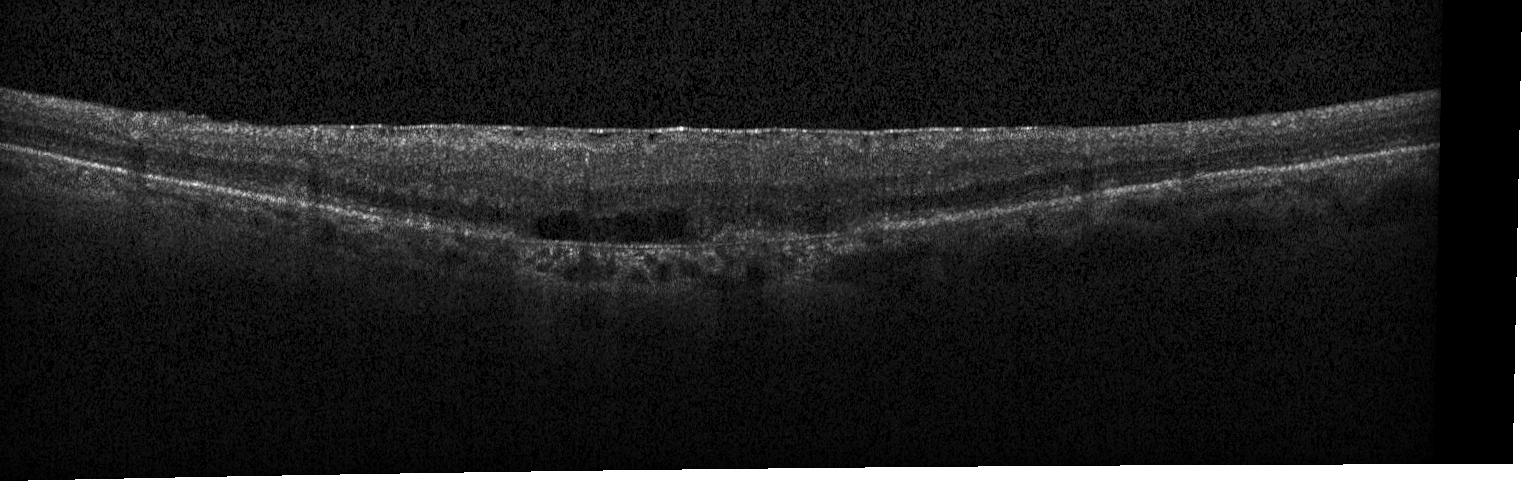

The scan shows a choroidal neovascular membrane.